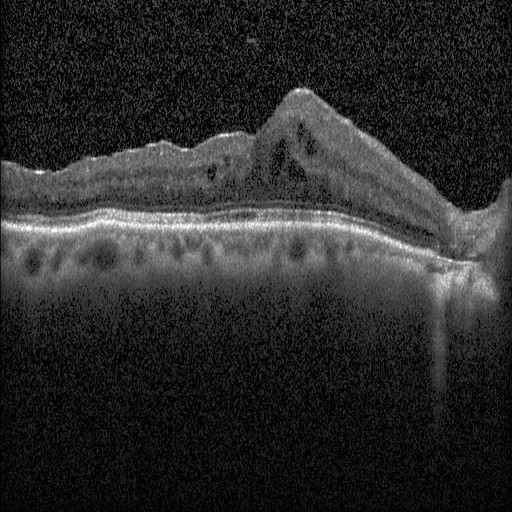
Macular OCT: diabetic macular edema.